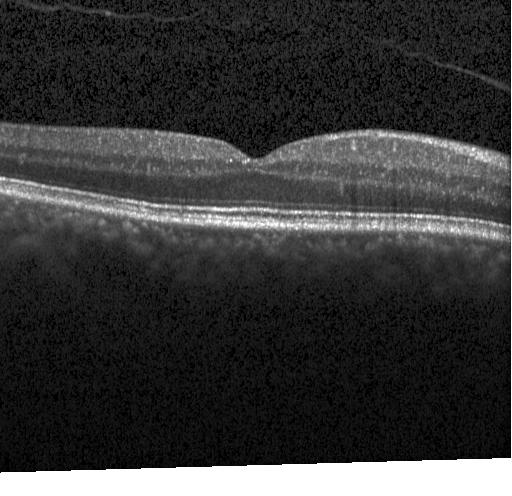 Acquired on a Heidelberg Spectralis · retinal OCT cross-section · spectral-domain OCT.
Assessment: neither CNV, DME, nor drusen.